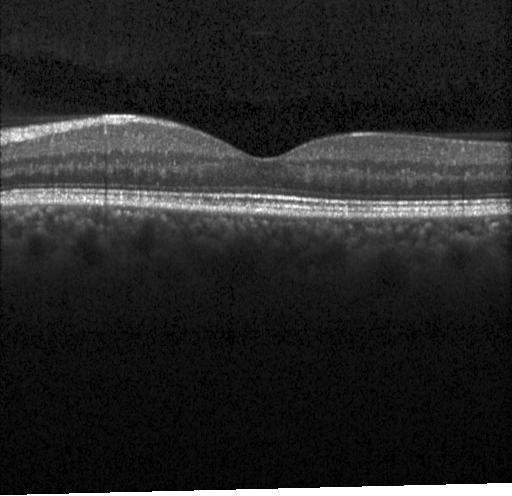 Retinal OCT cross-section · acquired on a Heidelberg Spectralis — Macular OCT: neither choroidal neovascularization, diabetic macular edema, nor drusen.